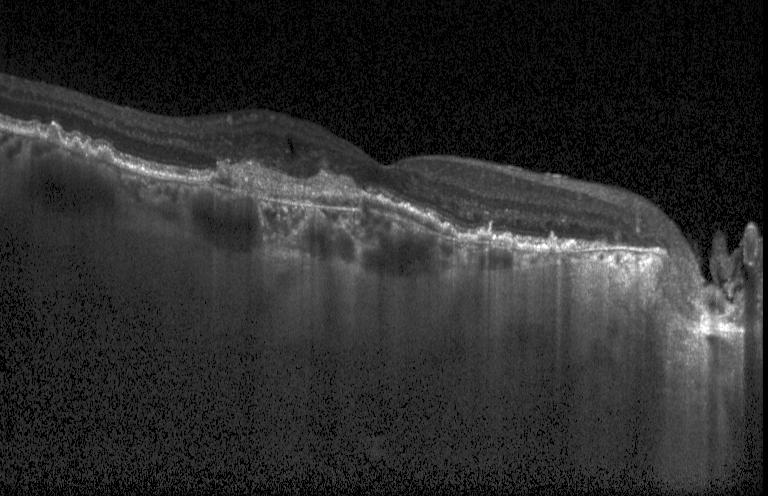
Spectral-domain OCT; fovea-centered; OCT B-scan.
Dx: a choroidal neovascular membrane.